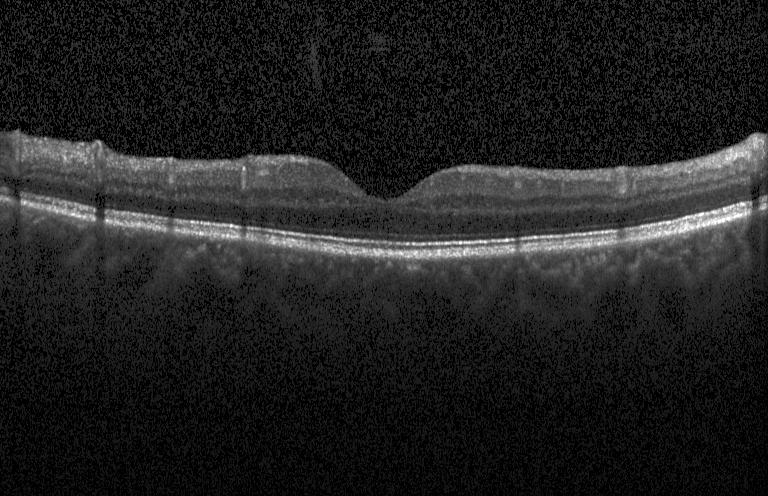 Retinal OCT cross-section — Finding: no evidence of choroidal neovascularization, diabetic macular edema, or drusen.